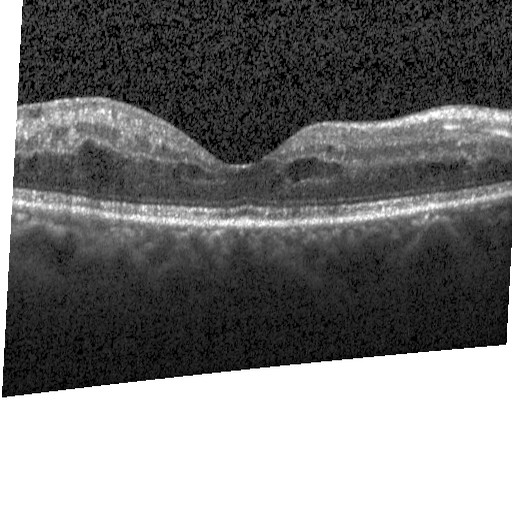

Macular OCT: DME.